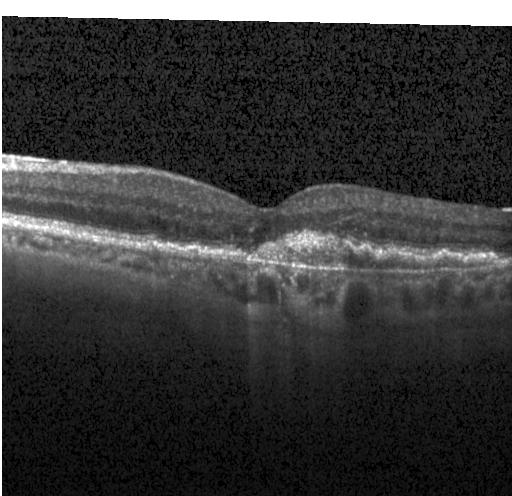
OCT line scan — The scan shows a choroidal neovascular membrane.